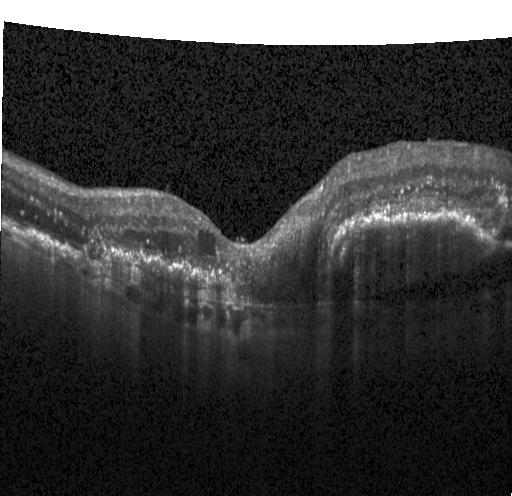
Heidelberg Spectralis, optical coherence tomography B-scan — Finding: a choroidal neovascular membrane.